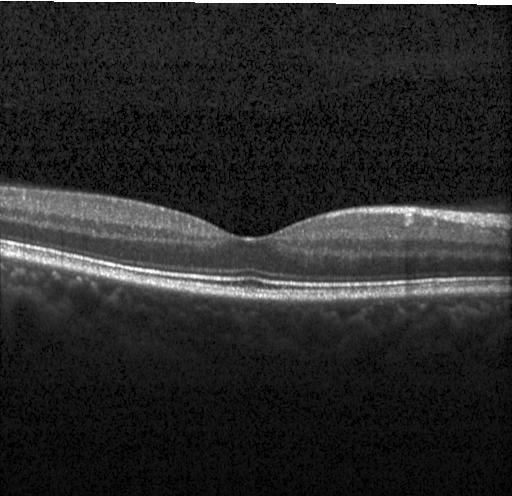

Retinal OCT cross-section — OCT finding: no evidence of CNV, DME, or drusen.